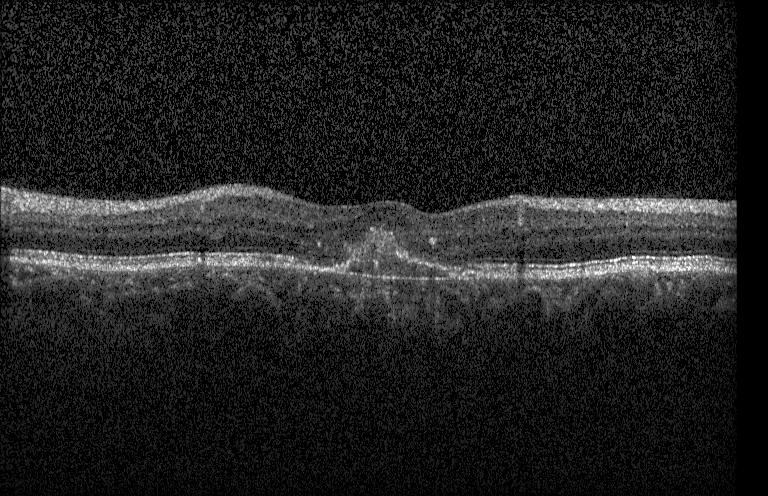
Macular OCT demonstrating choroidal neovascularization.